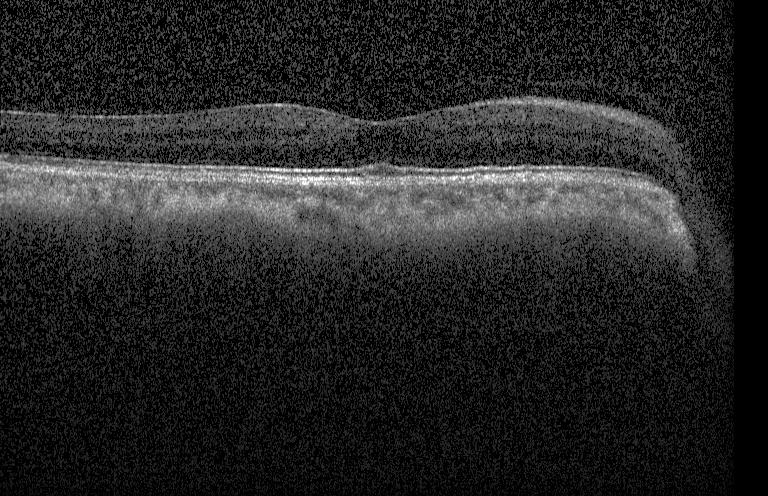
Instrument: Heidelberg Spectralis. Optical coherence tomography B-scan. Diagnosis: no CNV, DME, or drusen.